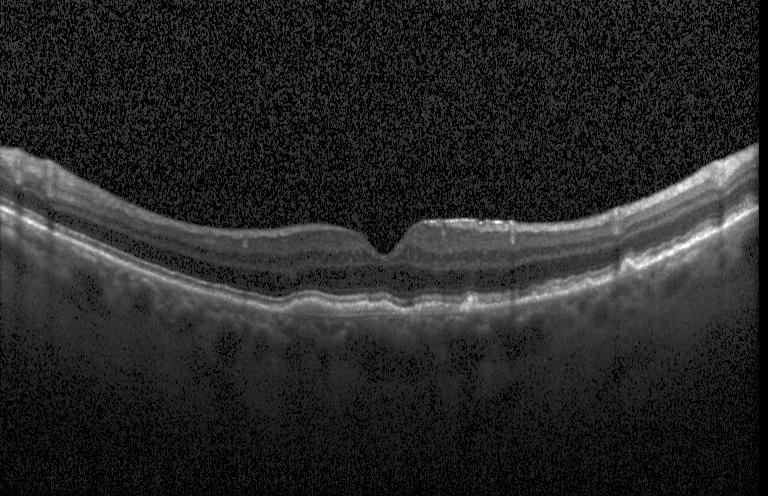
OCT line scan; fovea-centered; spectral-domain optical coherence tomography — Dx: CNV.